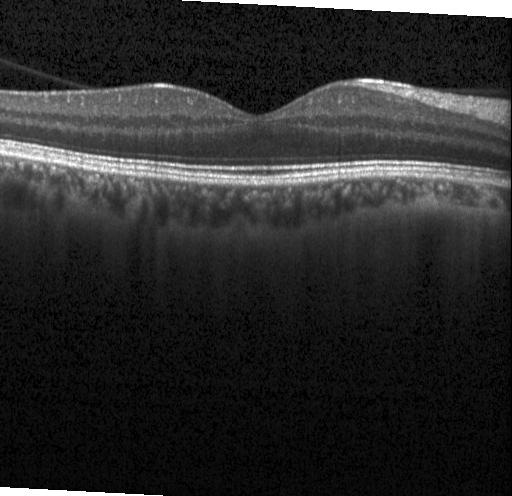
Diagnosis: no choroidal neovascularization, diabetic macular edema, or drusen.